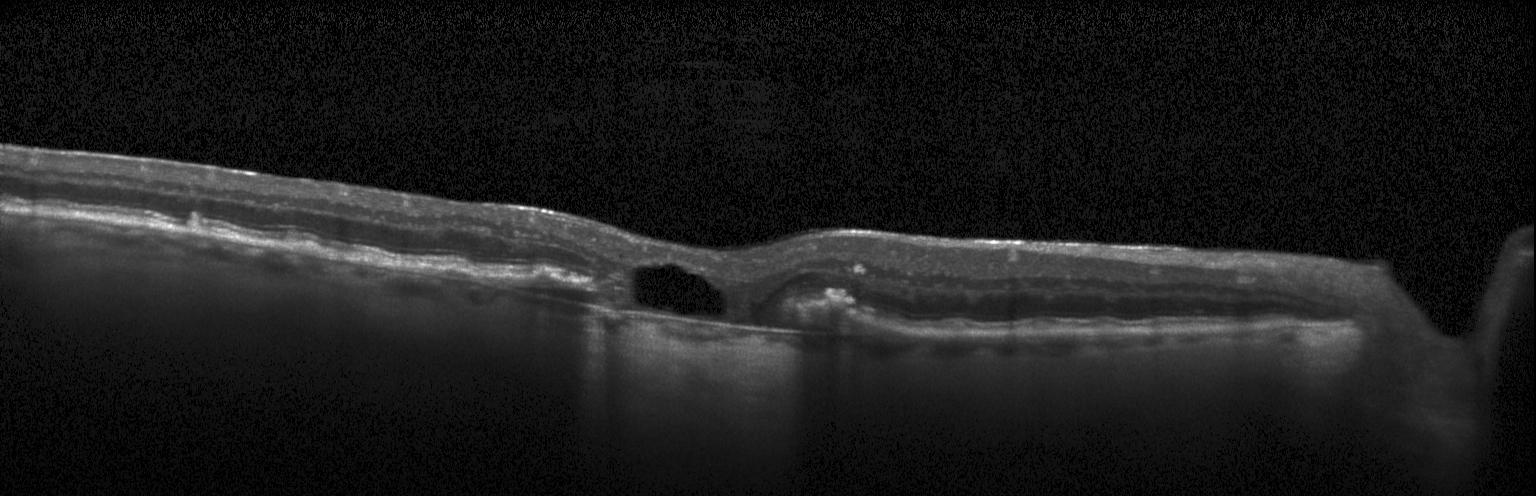 Dx: choroidal neovascularization.